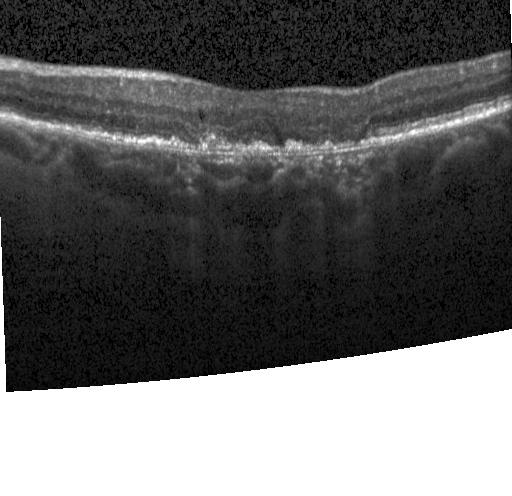 Horizontal scan through the fovea; optical coherence tomography scan; acquired on a Heidelberg Spectralis.
Finding: a choroidal neovascular membrane.